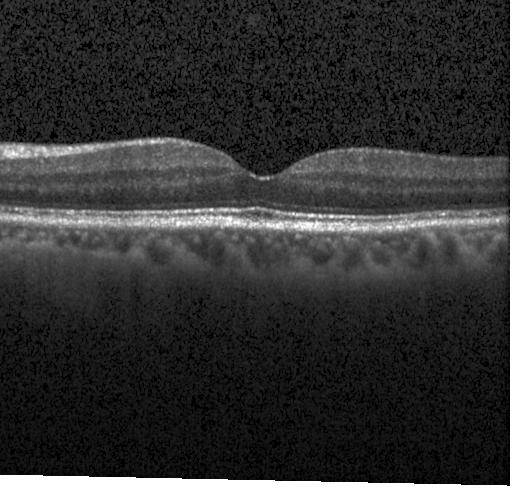 Neither choroidal neovascularization, diabetic macular edema, nor drusen.